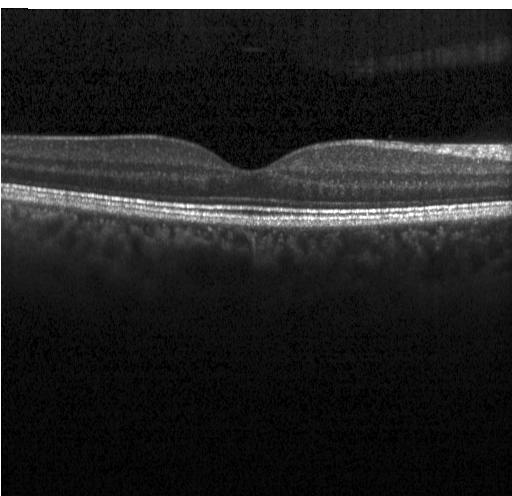

Macular scan. Optical coherence tomography scan.
Impression: no choroidal neovascularization, no diabetic macular edema, and no drusen.